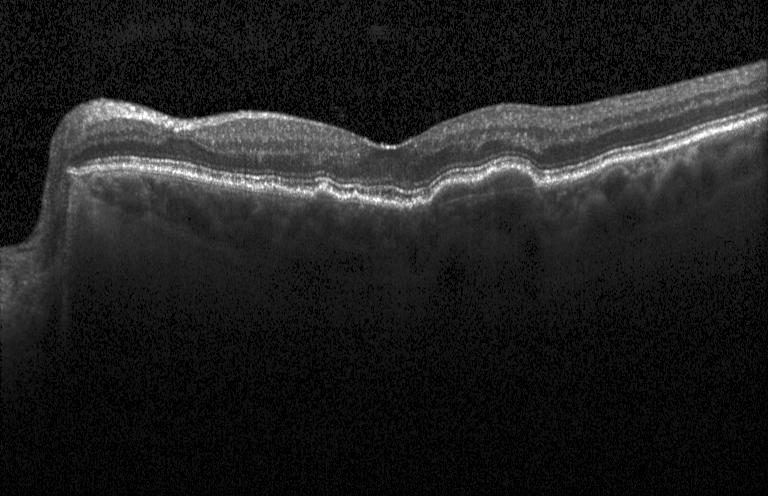 Retinal OCT B-scan. SD-OCT. Through the macula — Impression: a choroidal neovascular membrane.